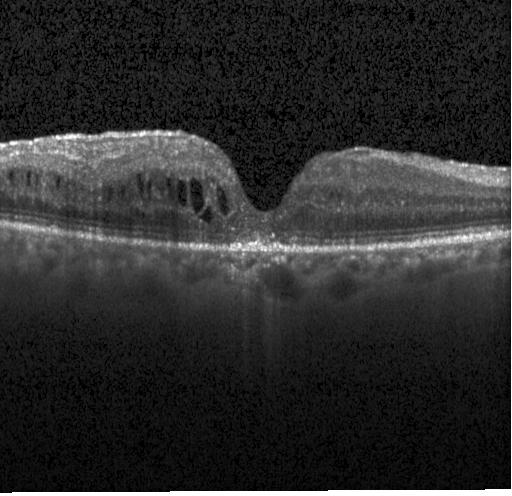

The scan shows diabetic macular edema.